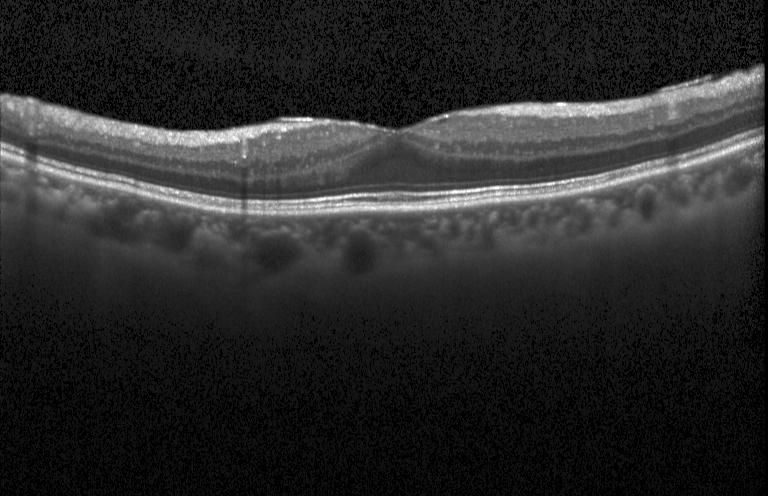 Fovea-centered, retinal OCT B-scan, Heidelberg Spectralis OCT system.
Finding: no CNV, DME, or drusen.